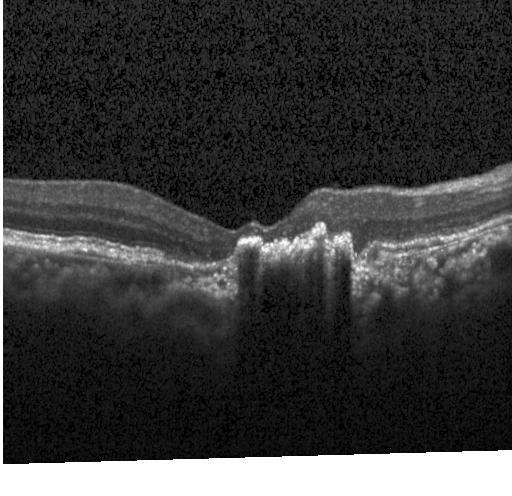 Spectral-domain OCT; retinal OCT B-scan.
The scan shows a choroidal neovascular membrane.